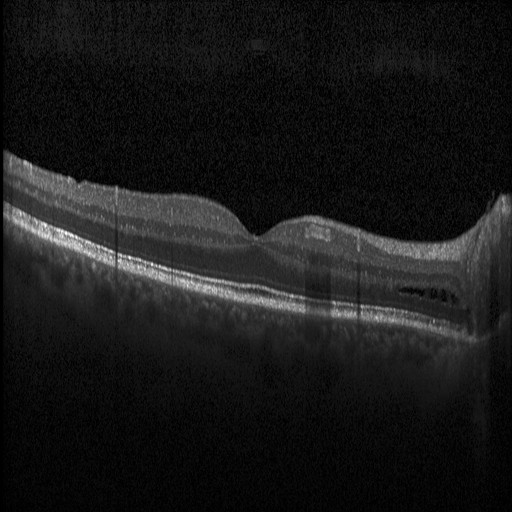
DME.